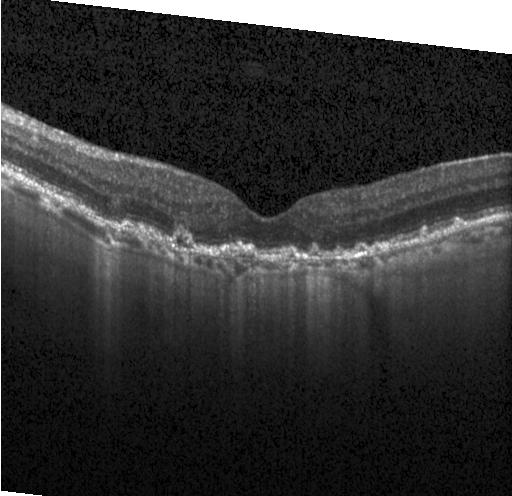

Fovea-centered · instrument: Heidelberg Spectralis · spectral-domain optical coherence tomography · retinal OCT B-scan.
This B-scan demonstrates choroidal neovascularization.